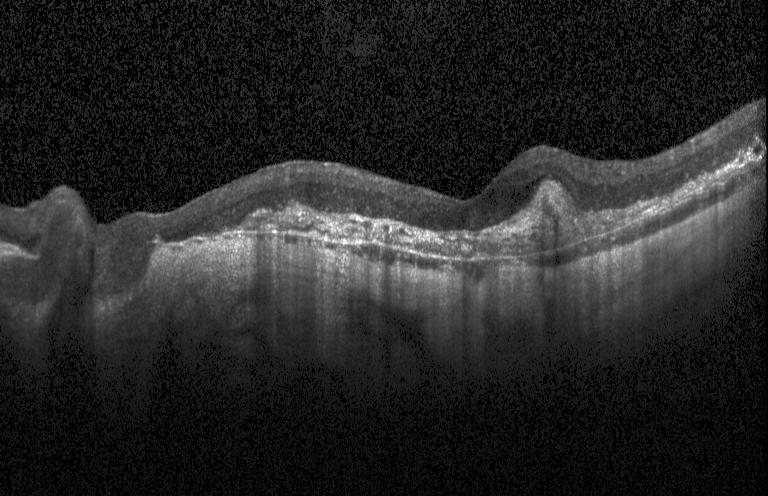
OCT B-scan showing choroidal neovascularization.